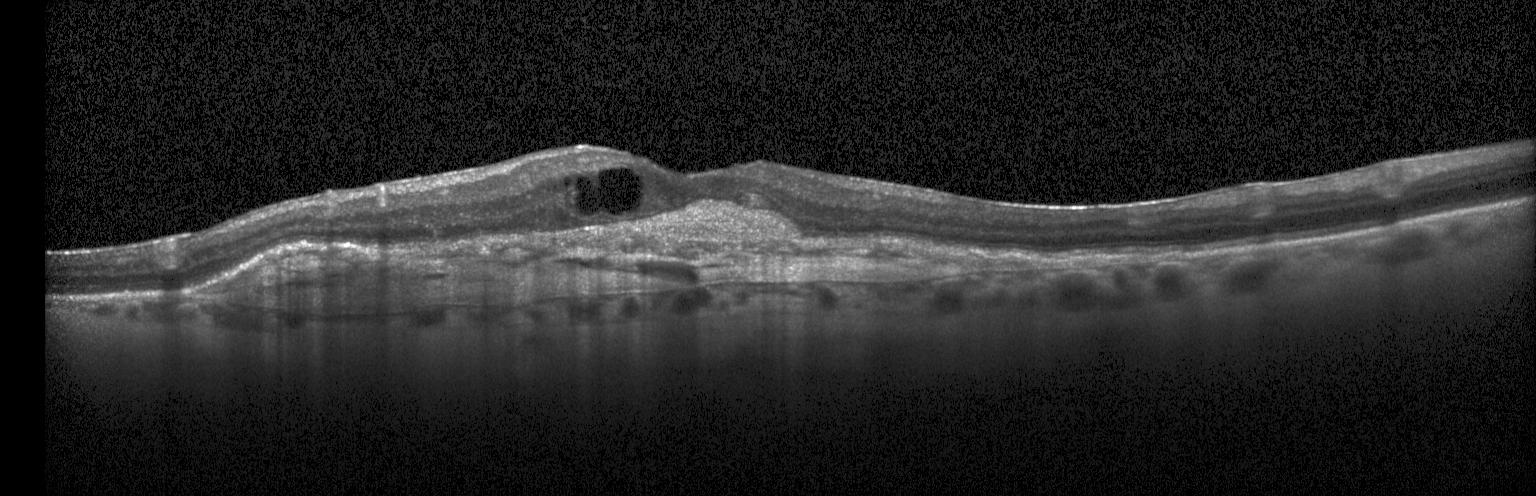

Optical coherence tomography B-scan; Heidelberg Spectralis
Finding: a choroidal neovascular membrane.